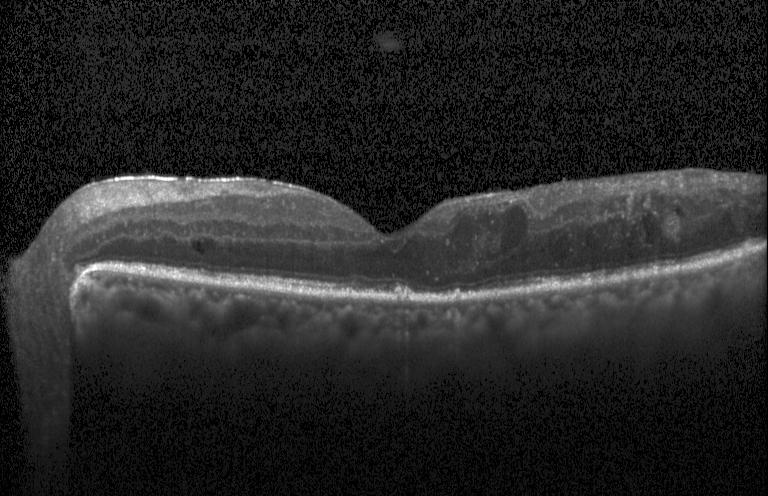 Impression: DME.